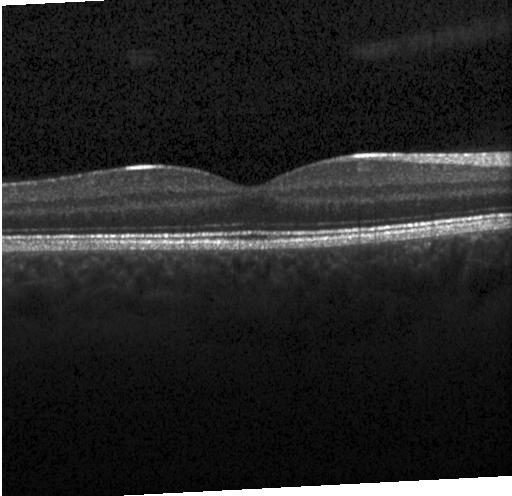
Macular OCT demonstrating no choroidal neovascularization, no diabetic macular edema, and no drusen.